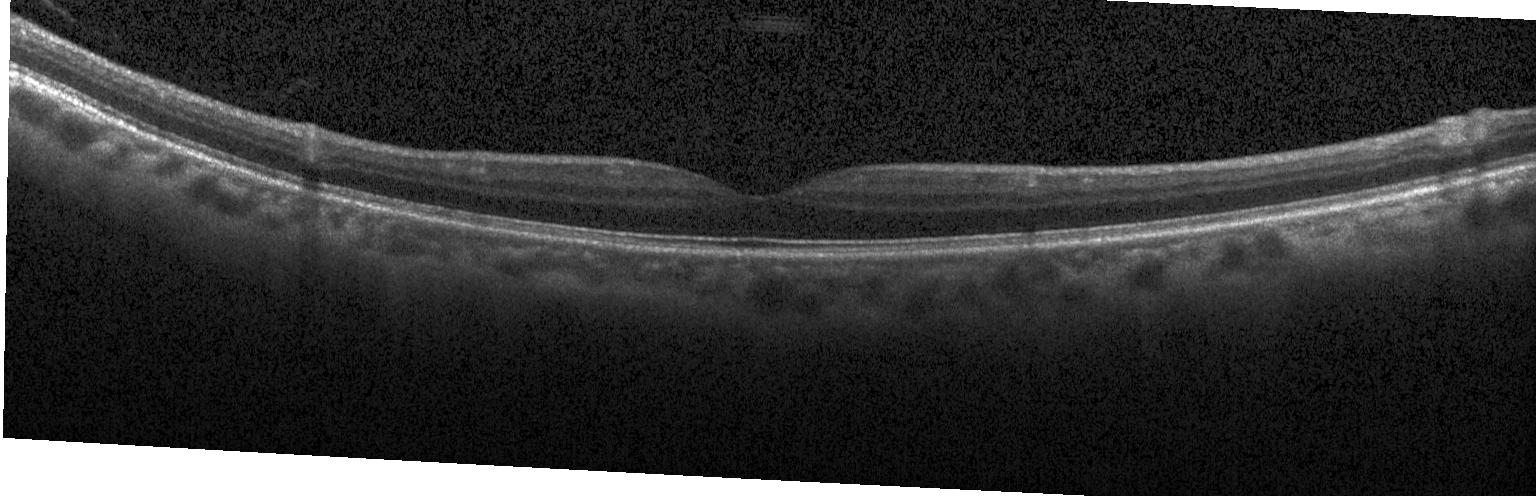
Heidelberg Spectralis. Retinal OCT cross-section. SD-OCT. Macular OCT: neither choroidal neovascularization, diabetic macular edema, nor drusen.